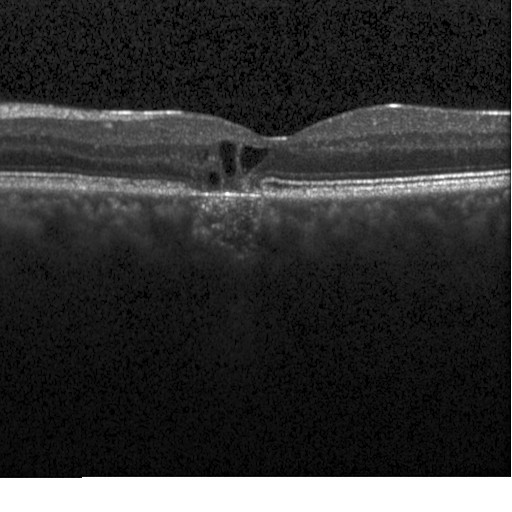 Retinal OCT cross-section showing DME.